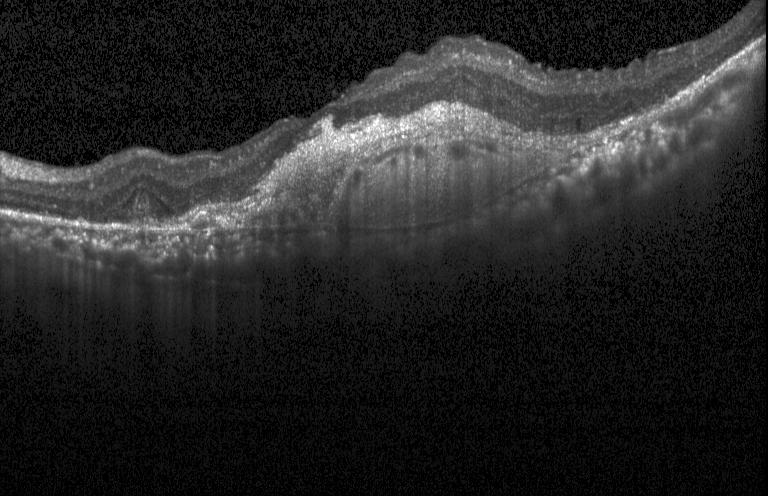

OCT B-scan · spectral-domain optical coherence tomography · Heidelberg Spectralis · fovea-centered — OCT finding: a choroidal neovascular membrane.